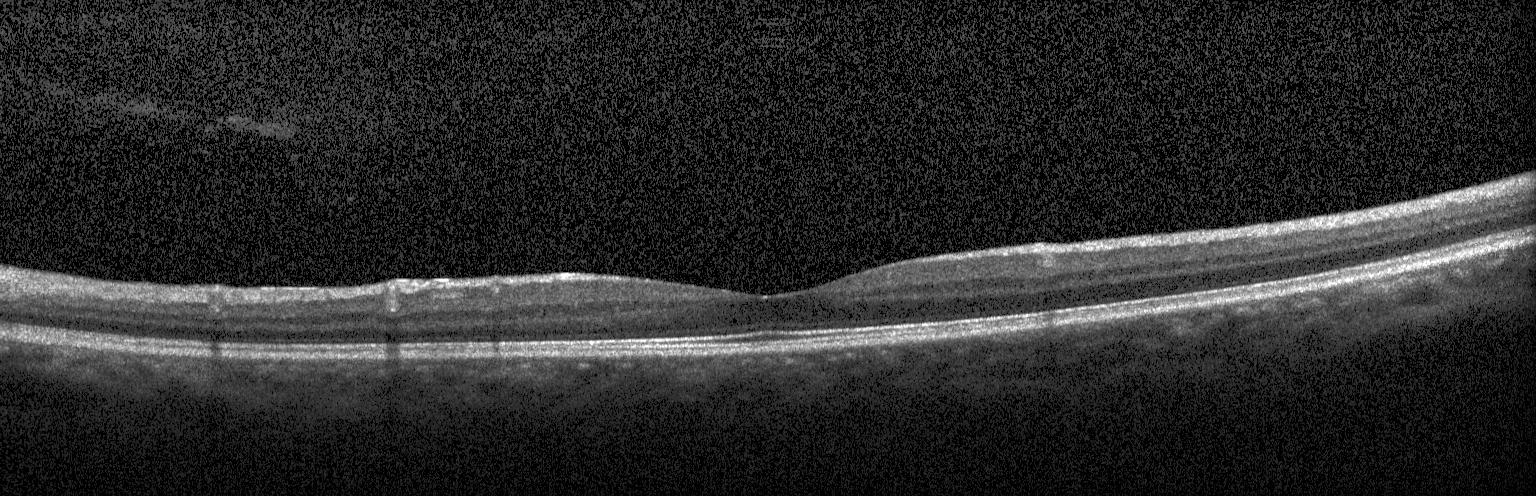 OCT scan showing no choroidal neovascularization, no diabetic macular edema, and no drusen.